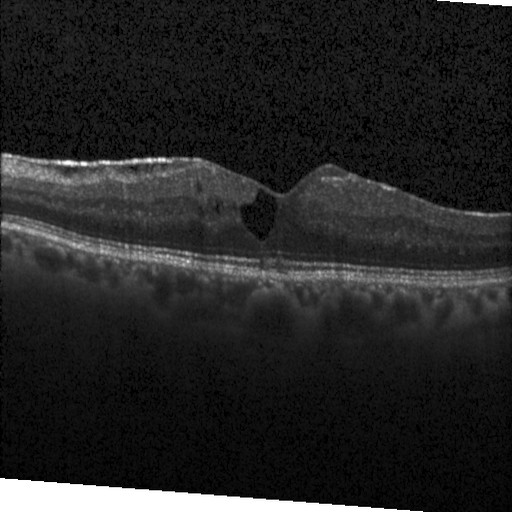

Diabetic macular edema.